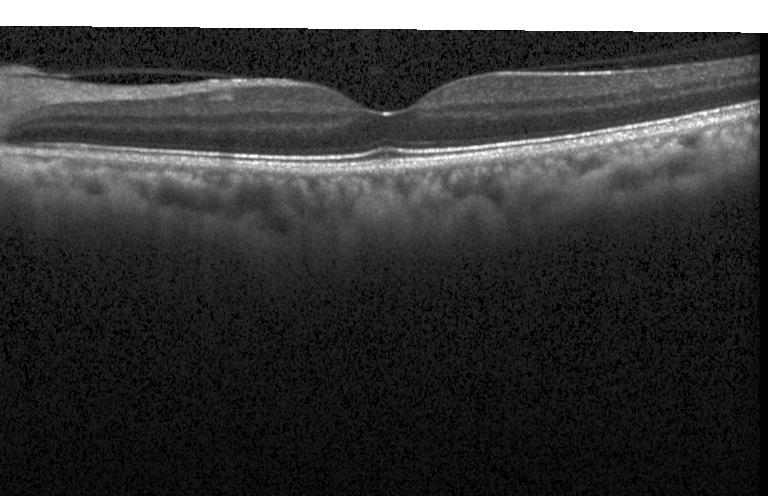 Fovea-centered. Instrument: Heidelberg Spectralis. Optical coherence tomography B-scan
No choroidal neovascularization, no diabetic macular edema, and no drusen.